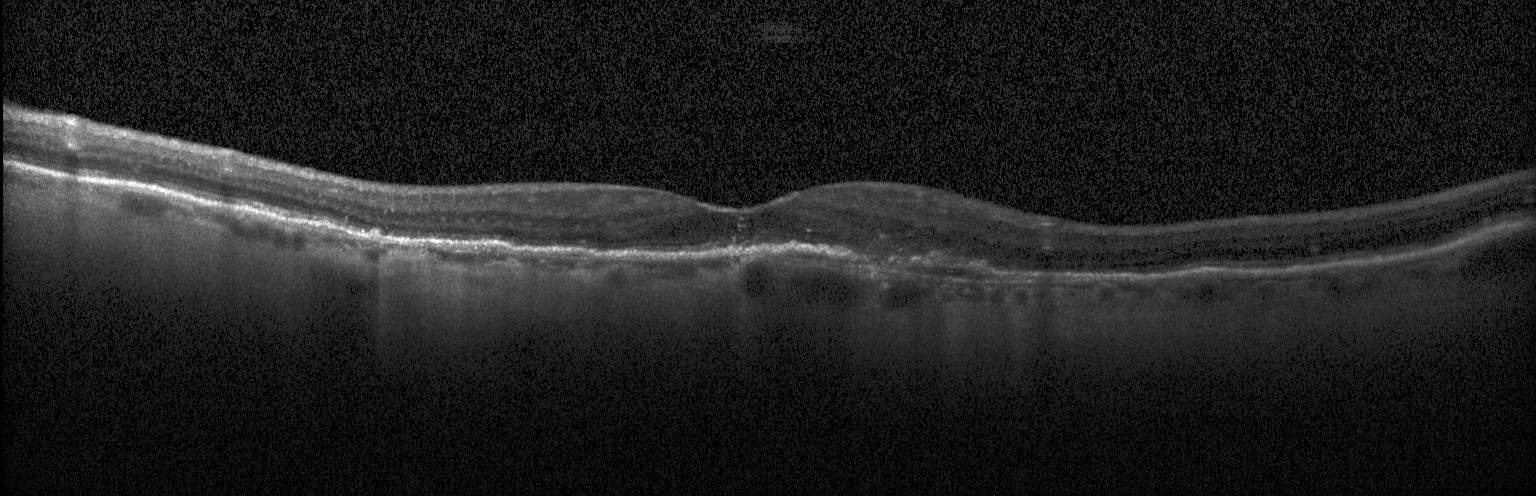

Macular scan · OCT line scan — Assessment: a choroidal neovascular membrane.